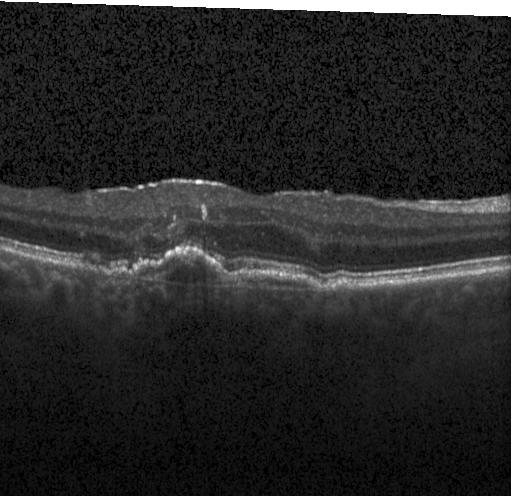

Macular OCT: a choroidal neovascular membrane.